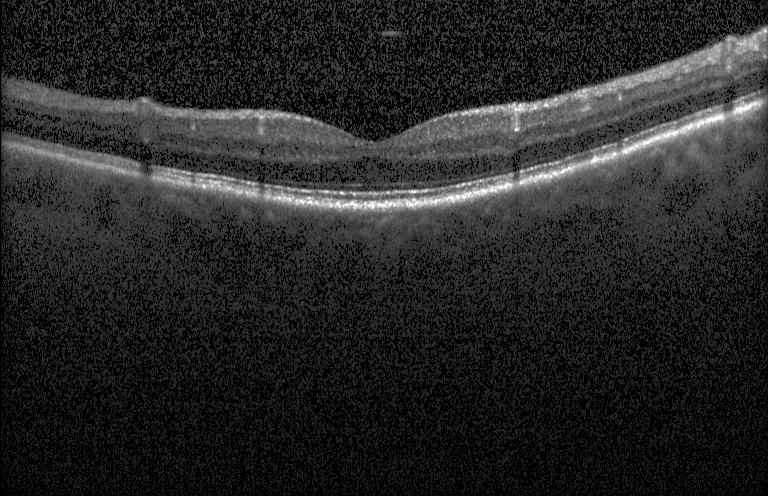 Retinal OCT B-scan · acquired on a Heidelberg Spectralis.
Impression: no choroidal neovascularization, diabetic macular edema, or drusen.